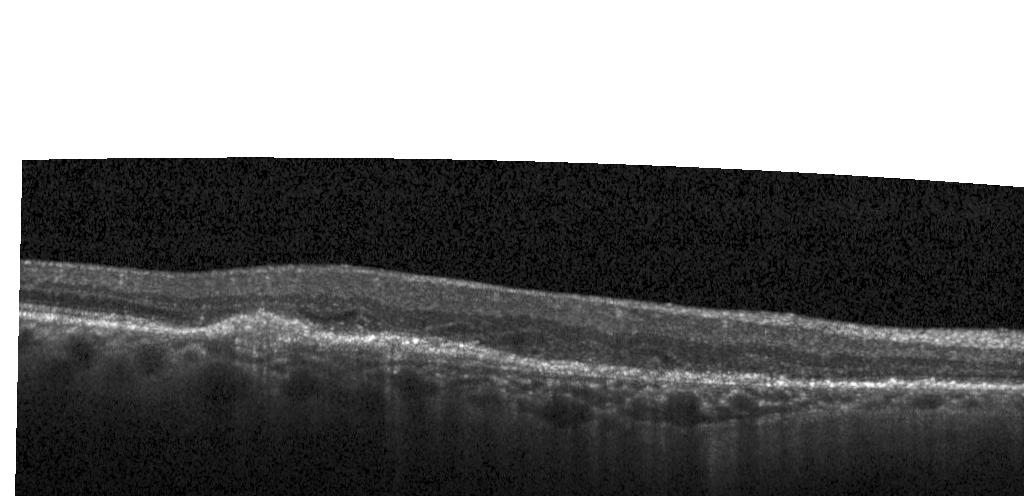 Spectral-domain OCT B-scan: choroidal neovascularization.